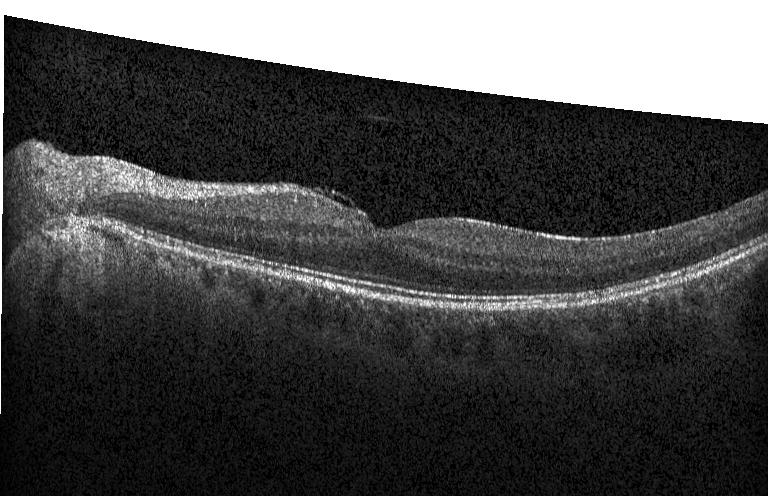 Spectral-domain OCT; Heidelberg Spectralis OCT system; retinal OCT cross-section; centered on the fovea.
Impression: no evidence of choroidal neovascularization, diabetic macular edema, or drusen.